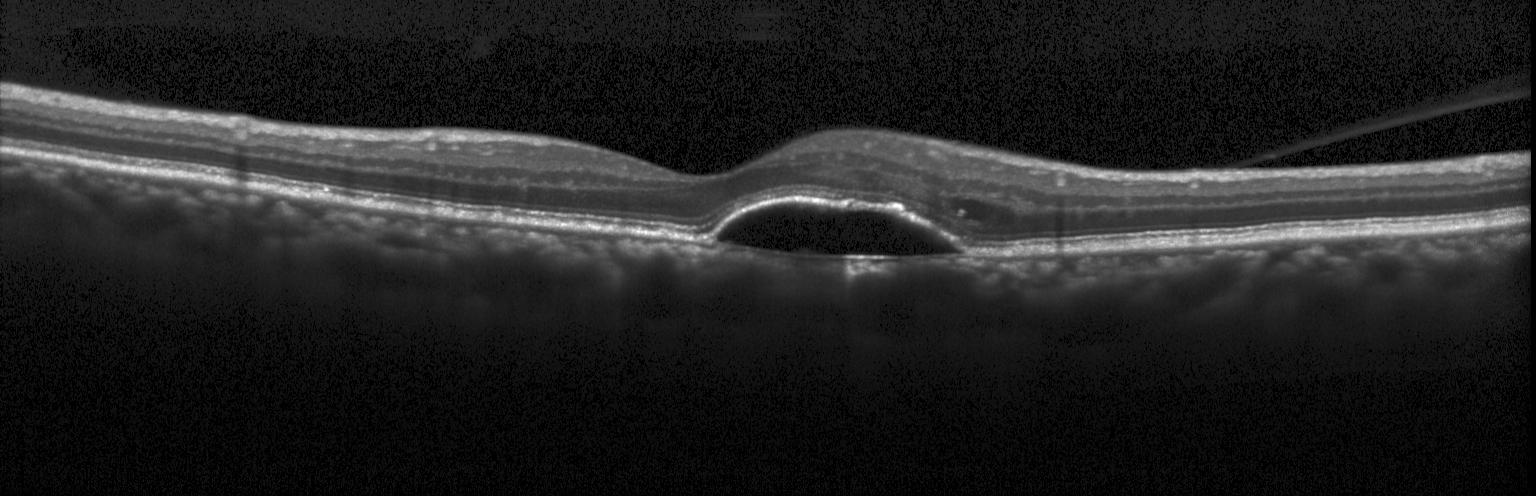 This B-scan demonstrates choroidal neovascularization (CNV).